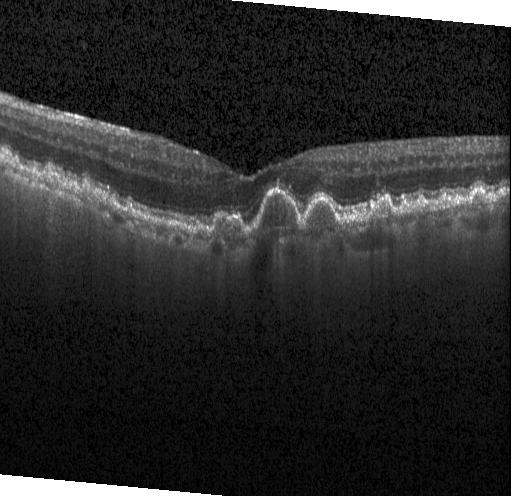
Finding: multiple drusen.